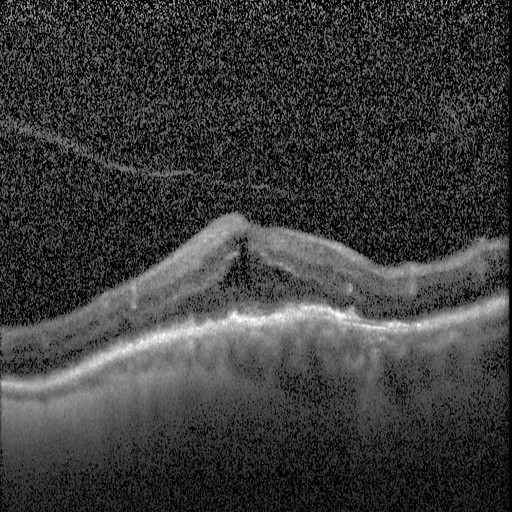

Macular scan; spectral-domain optical coherence tomography; Heidelberg Spectralis OCT system; optical coherence tomography B-scan — Dx: diabetic macular edema (DME).